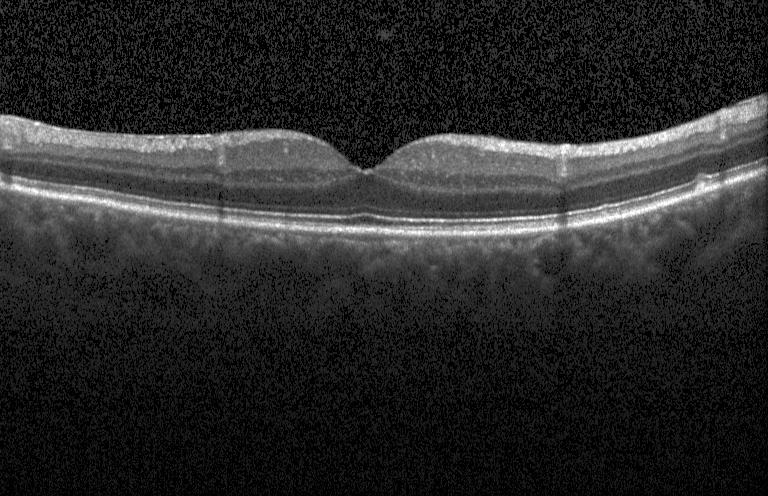
Instrument: Heidelberg Spectralis; OCT B-scan — Dx: multiple drusen.